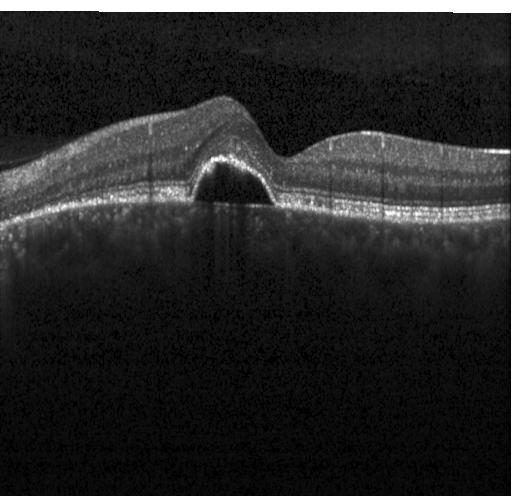
Spectral-domain OCT, centered on the fovea, retinal OCT B-scan — Assessment: a choroidal neovascular membrane.